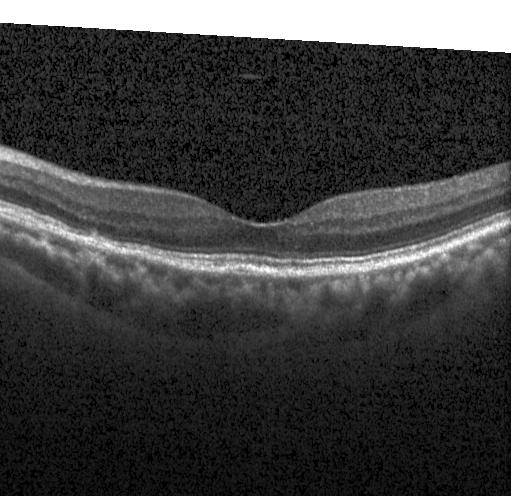
Fovea-centered. Optical coherence tomography scan. Instrument: Heidelberg Spectralis — Impression: no CNV, no DME, and no drusen.